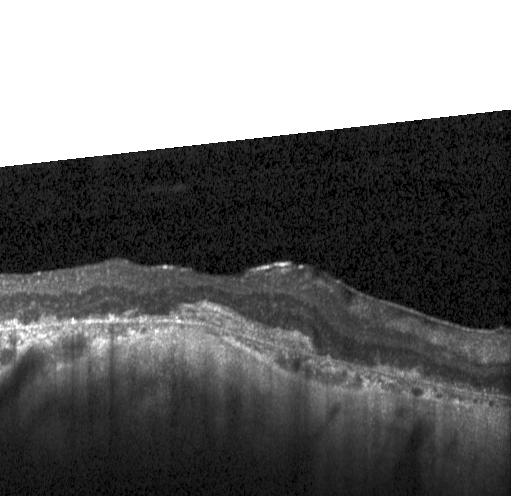
Optical coherence tomography B-scan.
Assessment: a choroidal neovascular membrane.